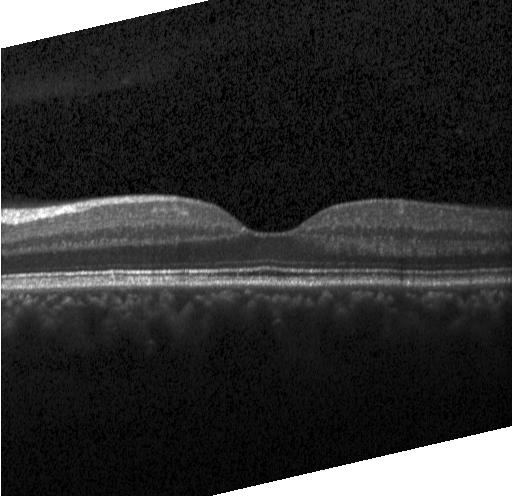 Retinal OCT B-scan. Spectral-domain OCT. Centered on the fovea. Acquired on a Heidelberg Spectralis.
Finding: no evidence of choroidal neovascularization, diabetic macular edema, or drusen.